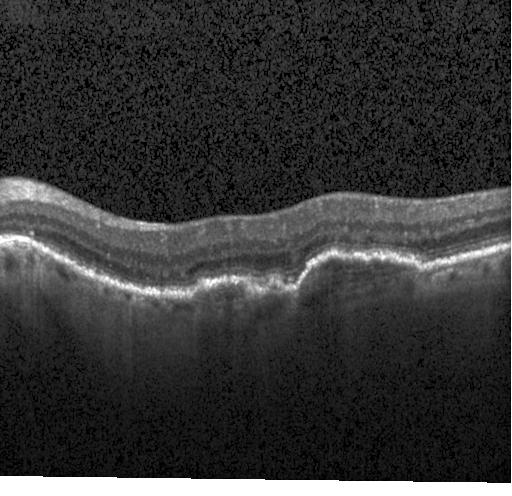

Spectral-domain OCT B-scan: a choroidal neovascular membrane.